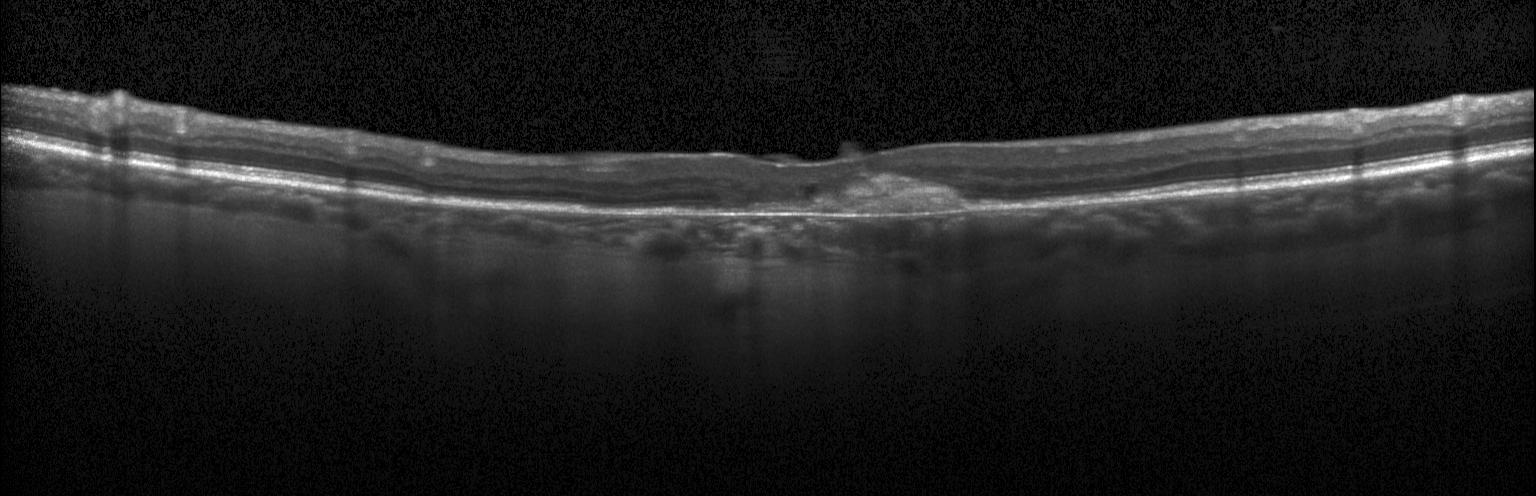
OCT B-scan, Heidelberg Spectralis, macular scan
A choroidal neovascular membrane.